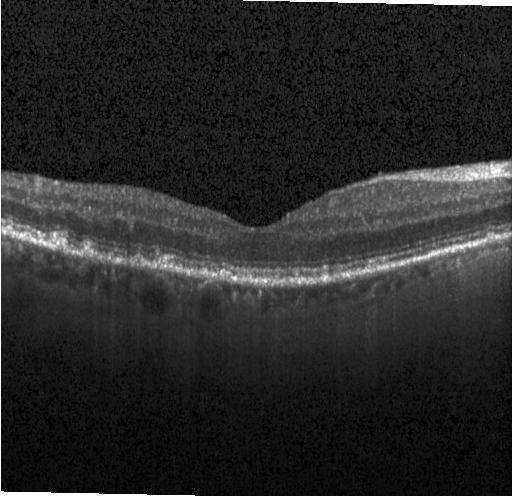

Impression: multiple drusen.